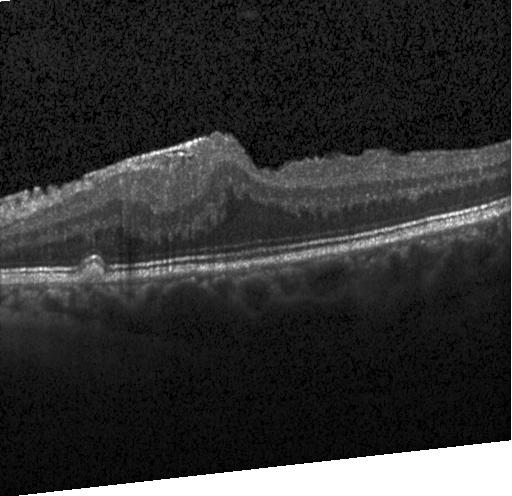
Optical coherence tomography B-scan
Assessment: drusen.